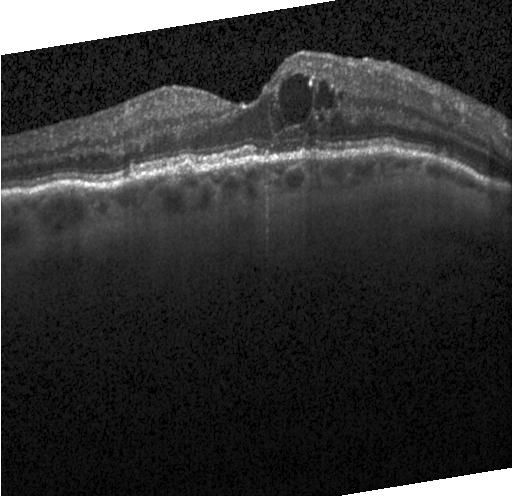

Horizontal scan through the fovea; OCT B-scan; acquired on a Heidelberg Spectralis.
This B-scan demonstrates a choroidal neovascular membrane.